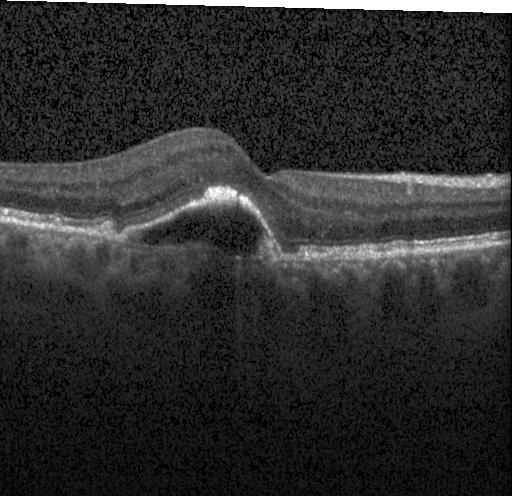 Through the macula · acquired on a Heidelberg Spectralis · OCT B-scan — Assessment: CNV.